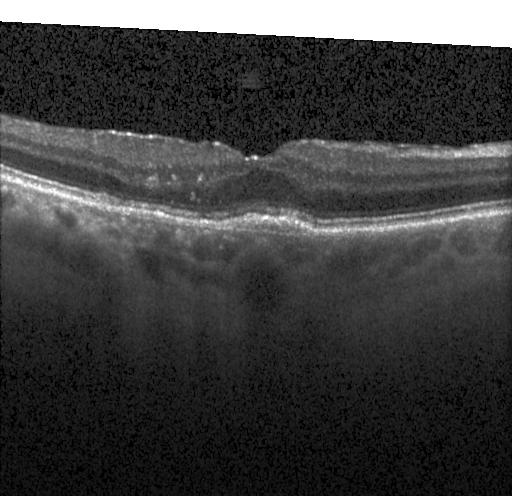

Dx: a choroidal neovascular membrane.